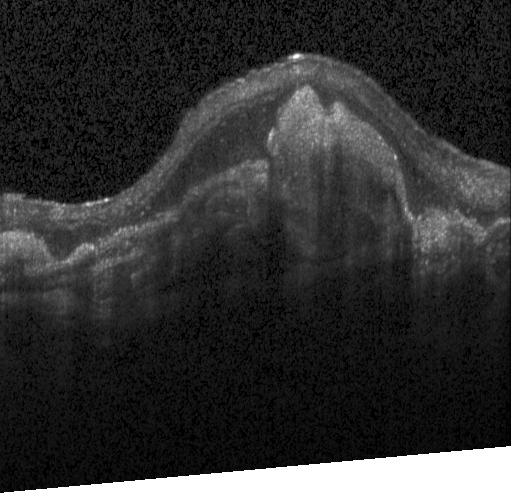
Retinal OCT B-scan; spectral-domain OCT; Heidelberg Spectralis
Finding: choroidal neovascularization.